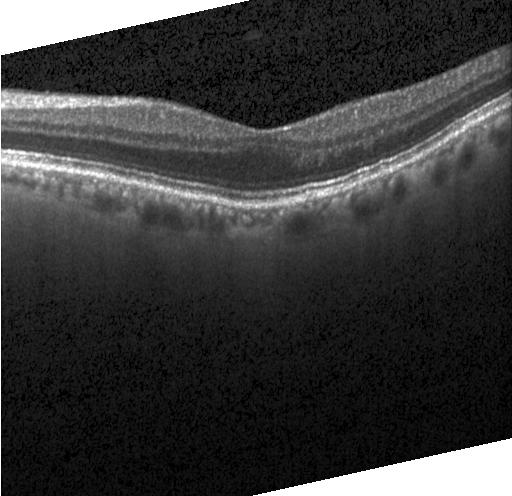 SD-OCT · optical coherence tomography B-scan
OCT finding: no CNV, no DME, and no drusen.